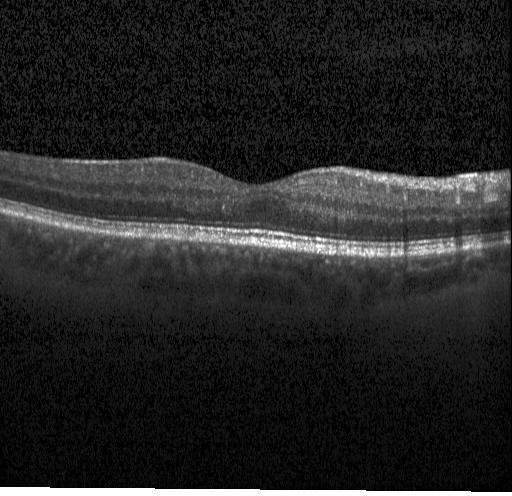
Dx: no choroidal neovascularization, no diabetic macular edema, and no drusen.